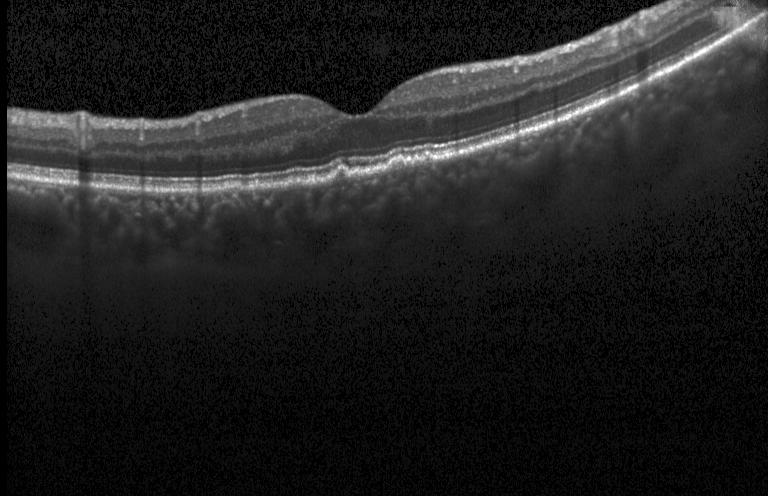
Diagnosis: drusen.